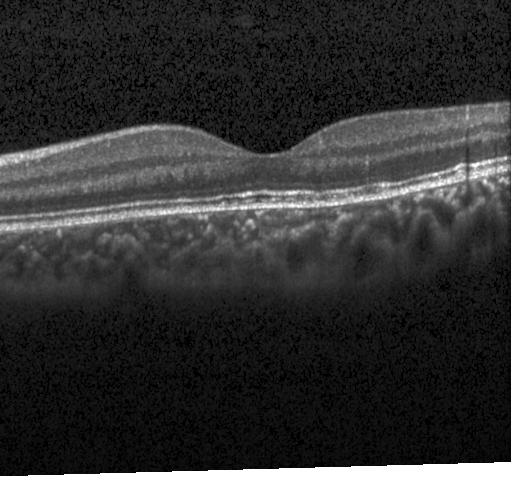
Horizontal scan through the fovea · OCT line scan · Heidelberg Spectralis. The scan shows neither CNV, DME, nor drusen.